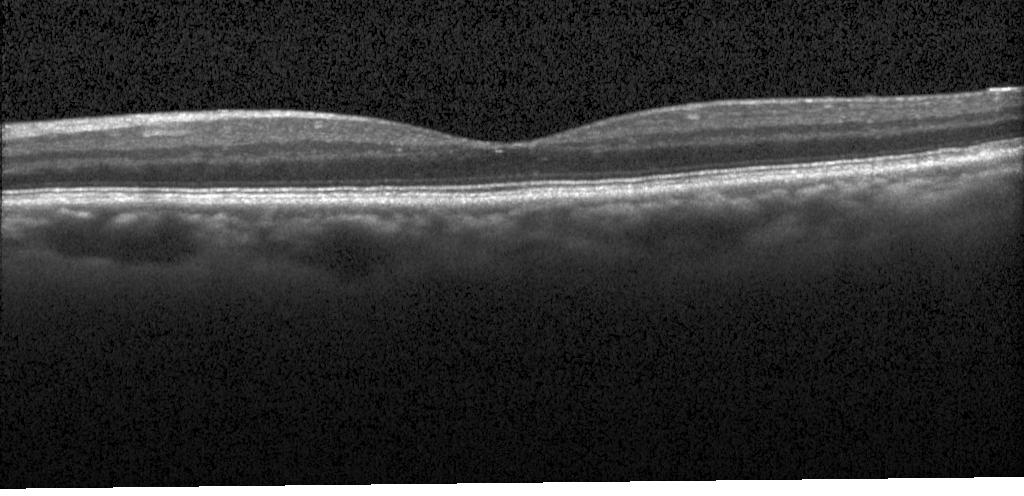 OCT finding: no evidence of CNV, DME, or drusen.